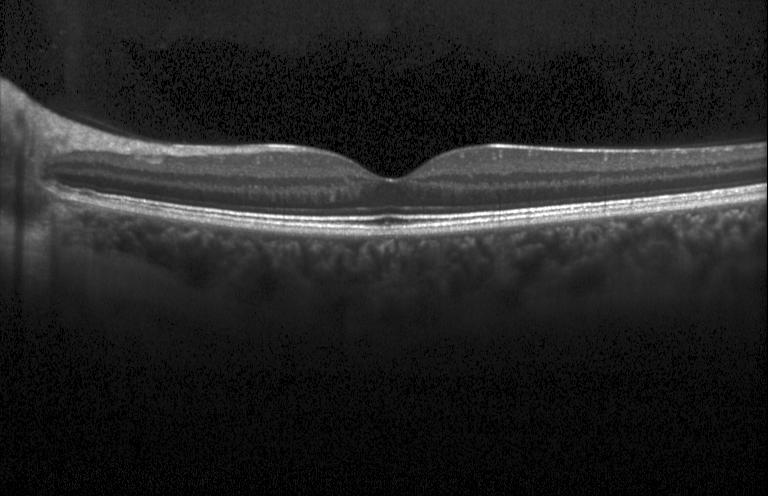 Finding: no evidence of choroidal neovascularization, diabetic macular edema, or drusen.